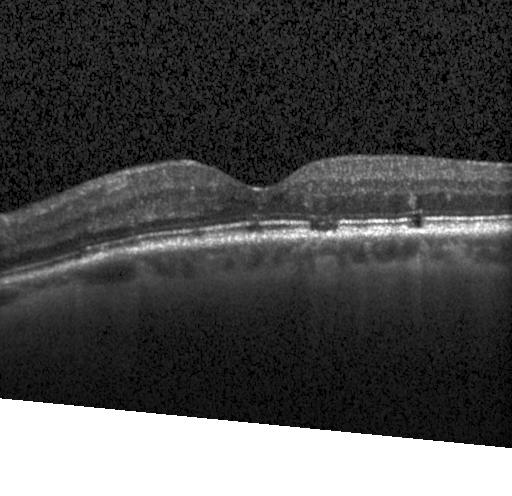
Heidelberg Spectralis OCT system; SD-OCT; OCT line scan; macular scan — Diabetic macular edema.